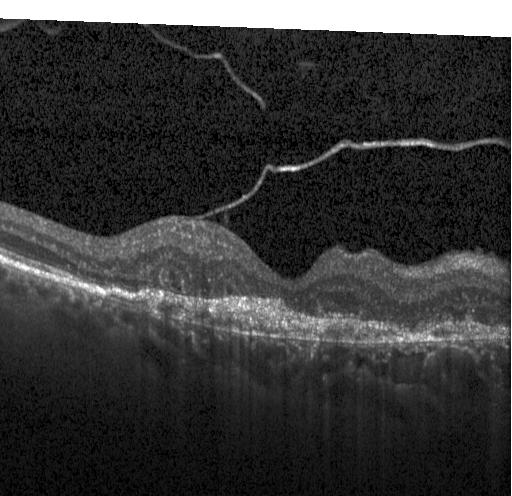
Acquired on a Heidelberg Spectralis, OCT B-scan, centered on the fovea — Finding: CNV.